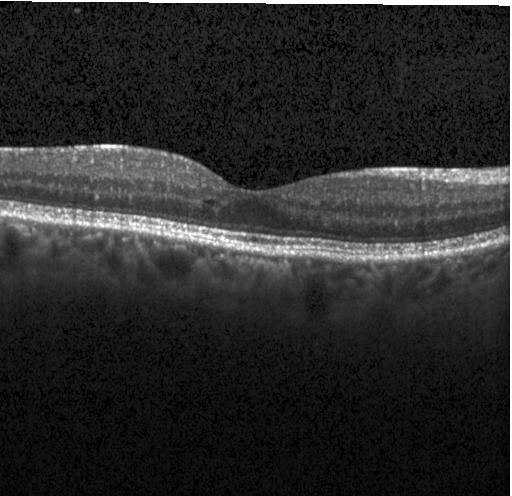

OCT B-scan showing no choroidal neovascularization, diabetic macular edema, or drusen.